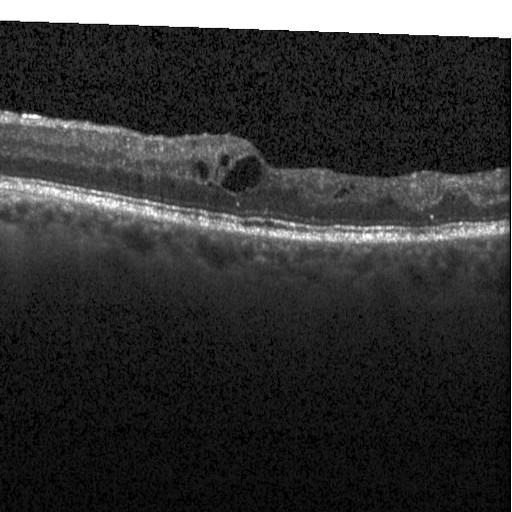 Finding: diabetic macular edema.